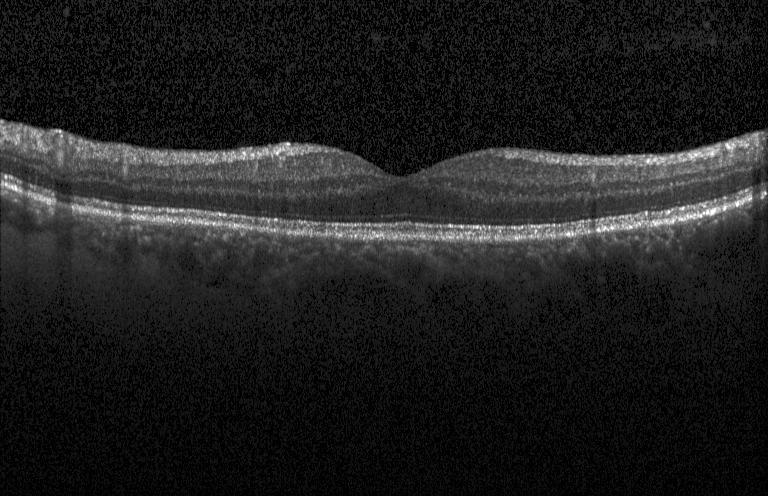

SD-OCT. Optical coherence tomography scan. Fovea-centered — Assessment: neither choroidal neovascularization, diabetic macular edema, nor drusen.